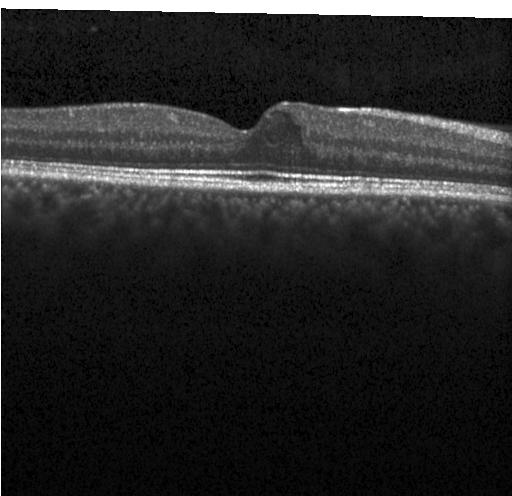 Horizontal scan through the fovea; OCT line scan; spectral-domain optical coherence tomography; acquired on a Heidelberg Spectralis.
Assessment: diabetic macular edema.